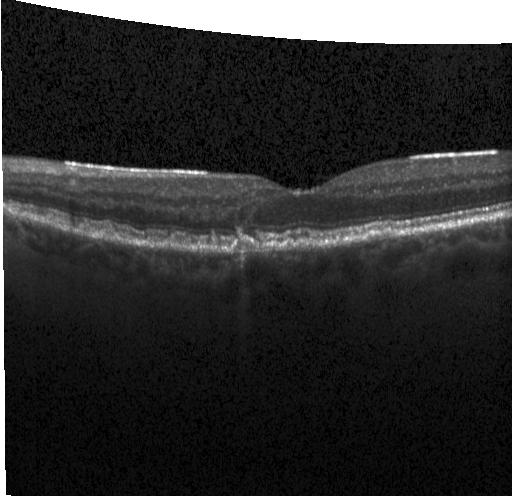

Retinal OCT cross-section, instrument: Heidelberg Spectralis, SD-OCT
The scan shows drusen.